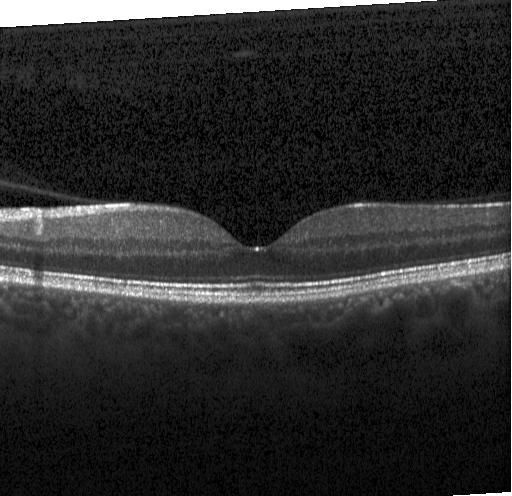
OCT B-scan, acquired on a Heidelberg Spectralis, macular scan. Finding: no CNV, no DME, and no drusen.